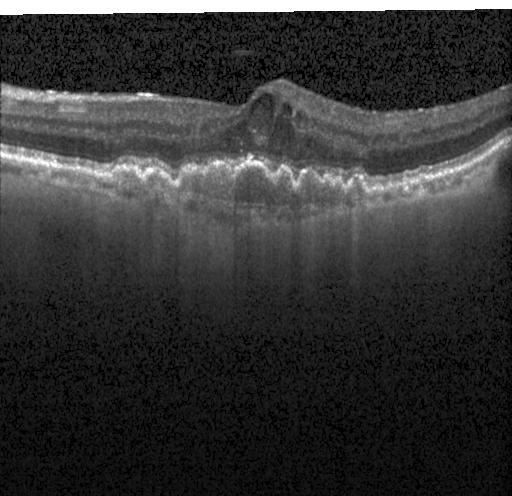

OCT B-scan.
Dx: a choroidal neovascular membrane.